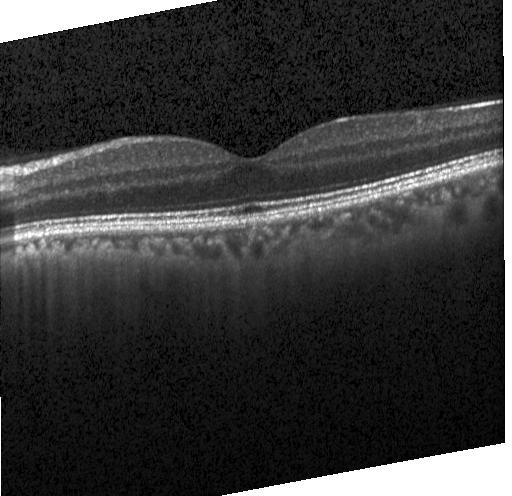
Diagnosis: no CNV, no DME, and no drusen.